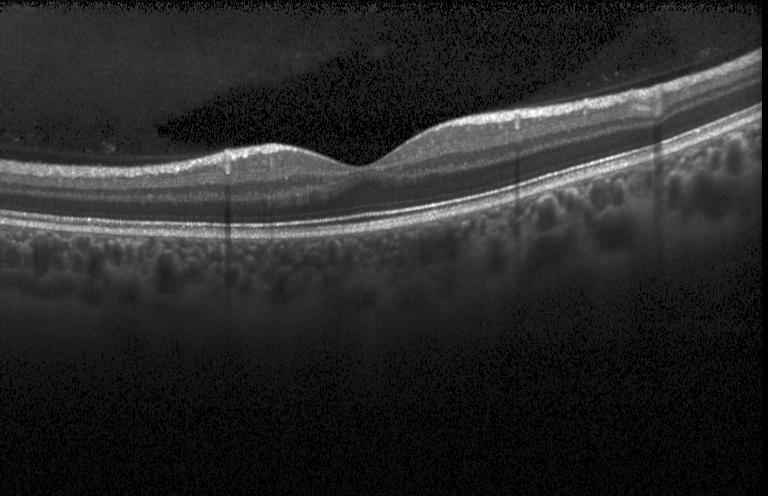 Optical coherence tomography B-scan. Centered on the fovea. Acquired on a Heidelberg Spectralis. Impression: no choroidal neovascularization, diabetic macular edema, or drusen.